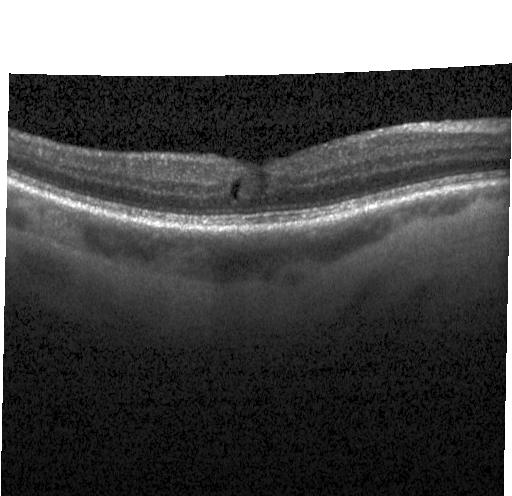 Finding: DME.